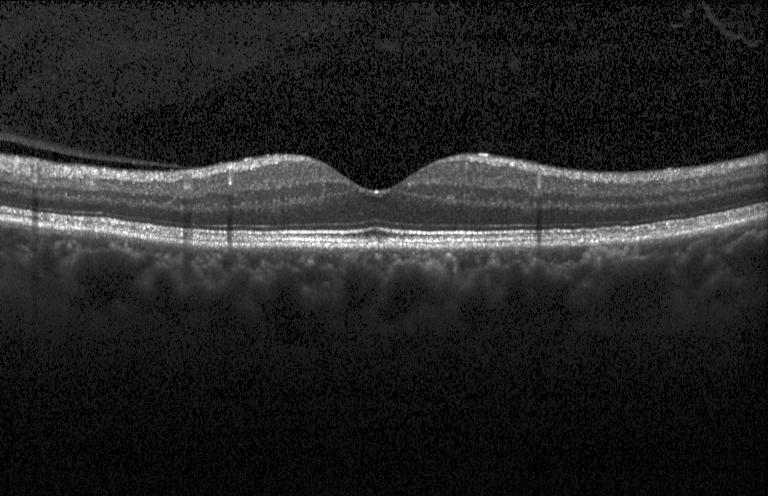 Retinal OCT B-scan. Macular scan. SD-OCT
This B-scan demonstrates no choroidal neovascularization, diabetic macular edema, or drusen.